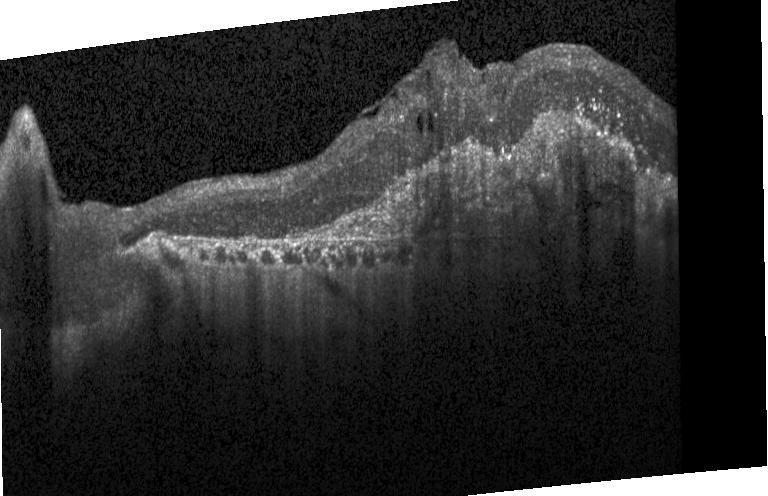 OCT finding: a choroidal neovascular membrane.